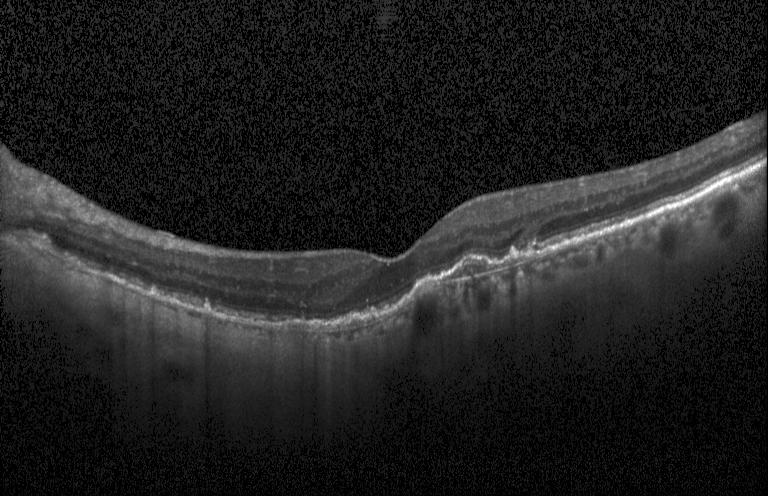

Instrument: Heidelberg Spectralis; retinal OCT B-scan — A choroidal neovascular membrane.